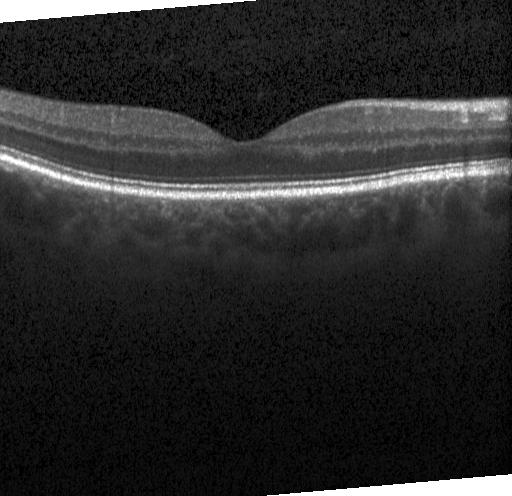
Heidelberg Spectralis OCT system, macular scan, retinal OCT B-scan. Dx: no evidence of choroidal neovascularization, diabetic macular edema, or drusen.